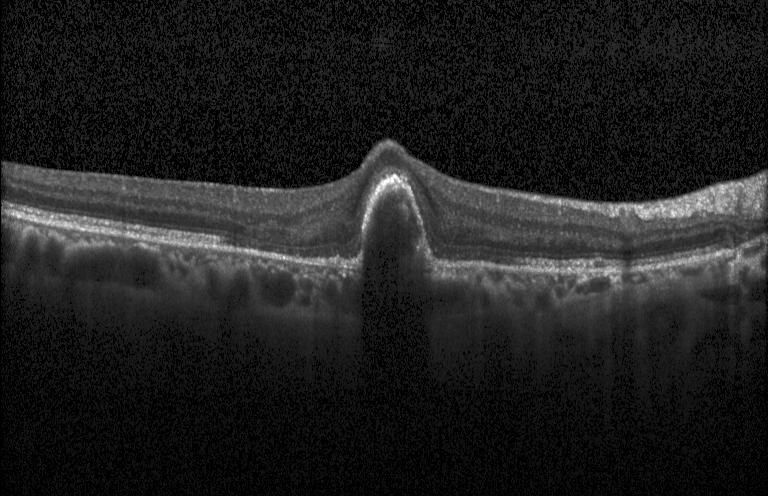
Optical coherence tomography B-scan
Impression: a choroidal neovascular membrane.